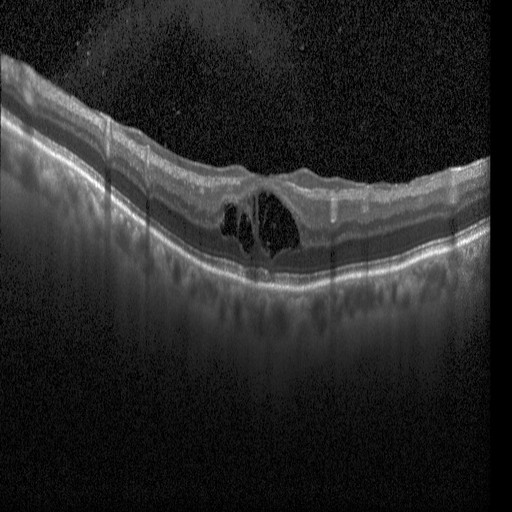 Finding: diabetic macular edema (DME).